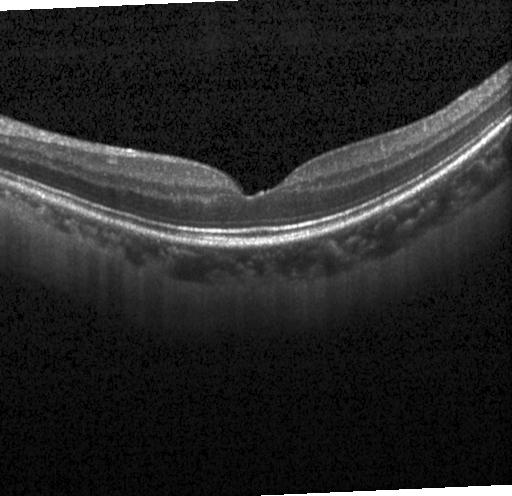 Dx: no CNV, no DME, and no drusen.